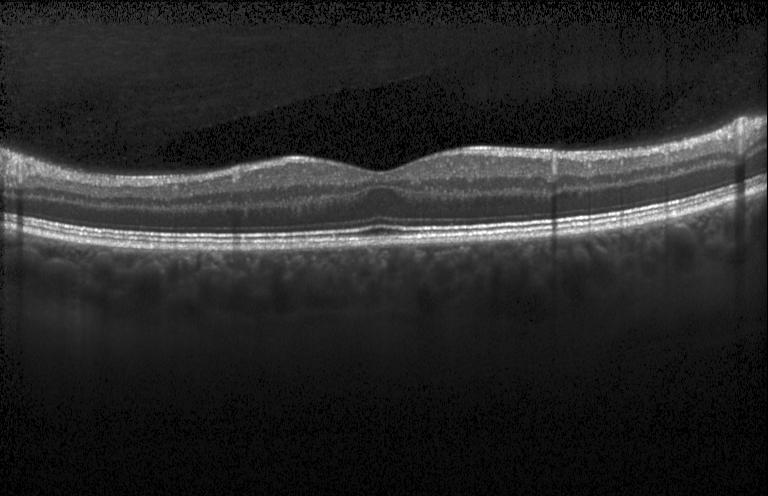
Retinal OCT cross-section. Dx: neither choroidal neovascularization, diabetic macular edema, nor drusen.